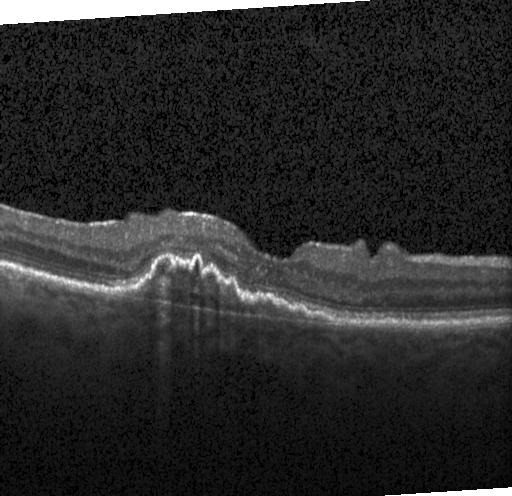
Retinal OCT cross-section, Heidelberg Spectralis — OCT finding: a choroidal neovascular membrane.